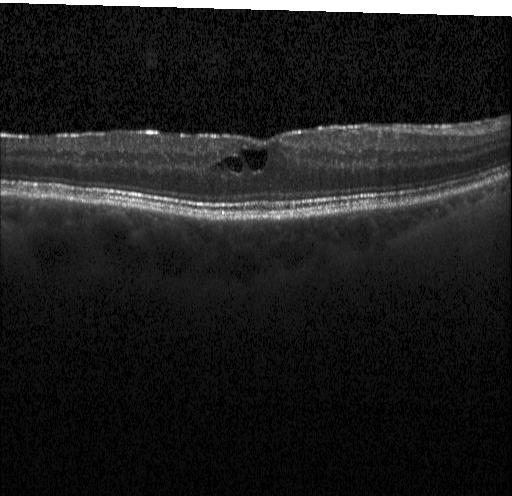

Finding: diabetic macular edema (DME).